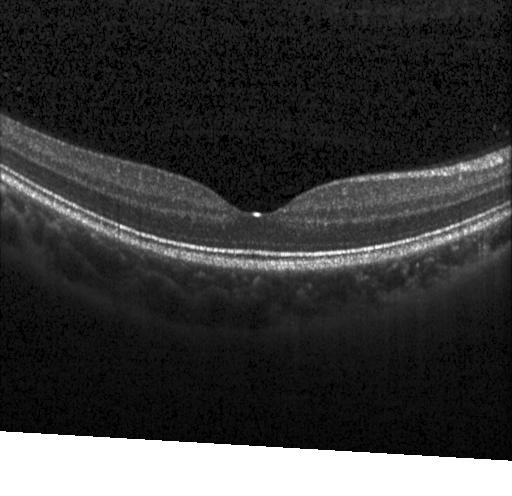 Optical coherence tomography scan. Diagnosis: no choroidal neovascularization, diabetic macular edema, or drusen.